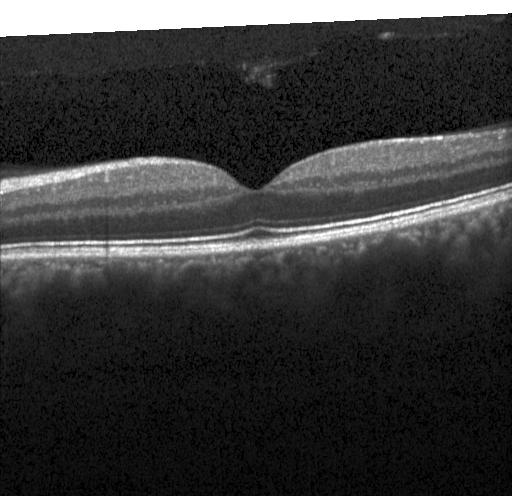

SD-OCT. Horizontal scan through the fovea. Retinal OCT B-scan — Diagnosis: no choroidal neovascularization, no diabetic macular edema, and no drusen.